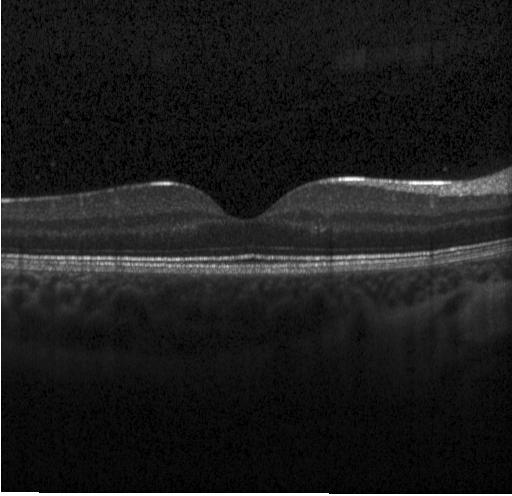 SD-OCT, retinal OCT cross-section — No evidence of CNV, DME, or drusen.